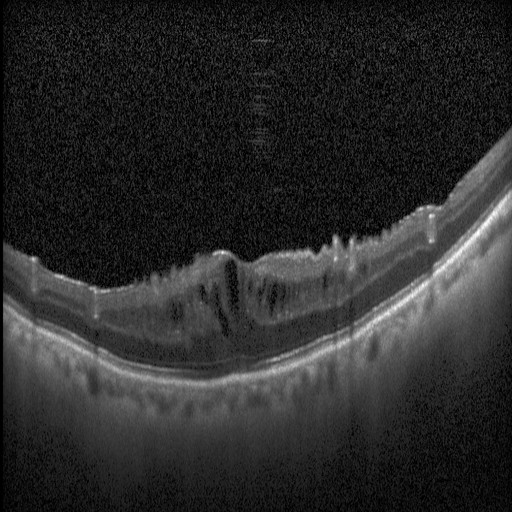

Diagnosis: DME.